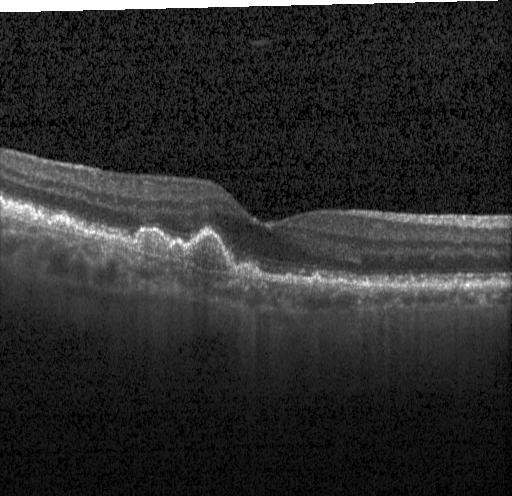
OCT line scan. Assessment: drusen.